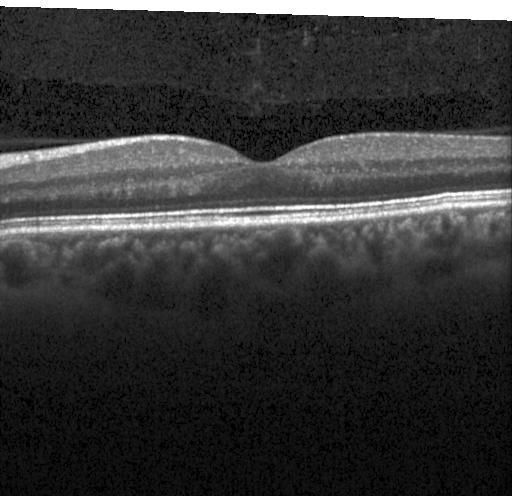
Optical coherence tomography scan. The scan shows no evidence of choroidal neovascularization, diabetic macular edema, or drusen.